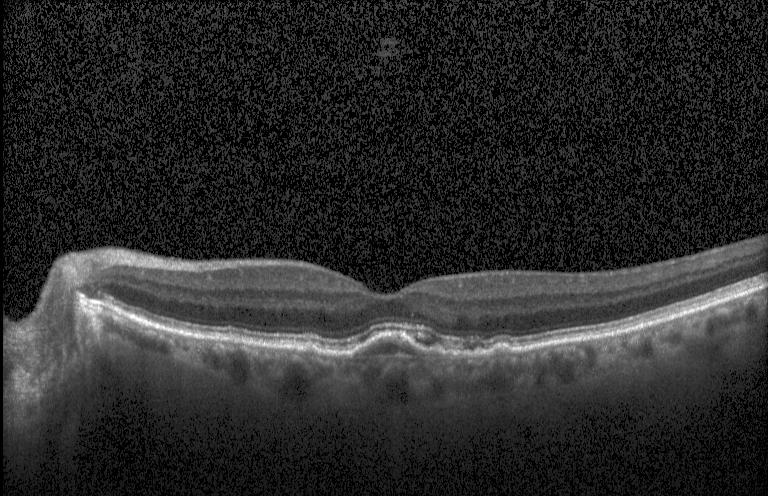

OCT B-scan — Finding: CNV.